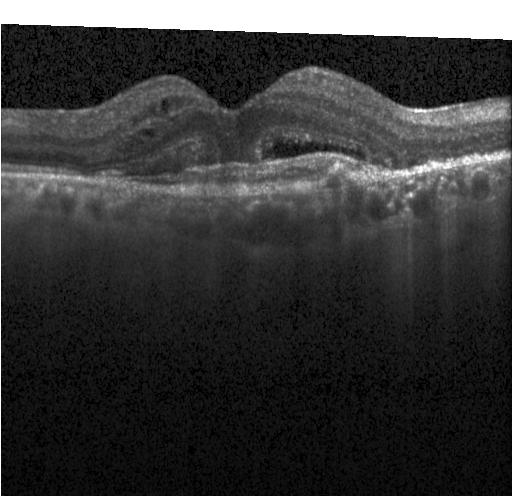

Finding: choroidal neovascularization.